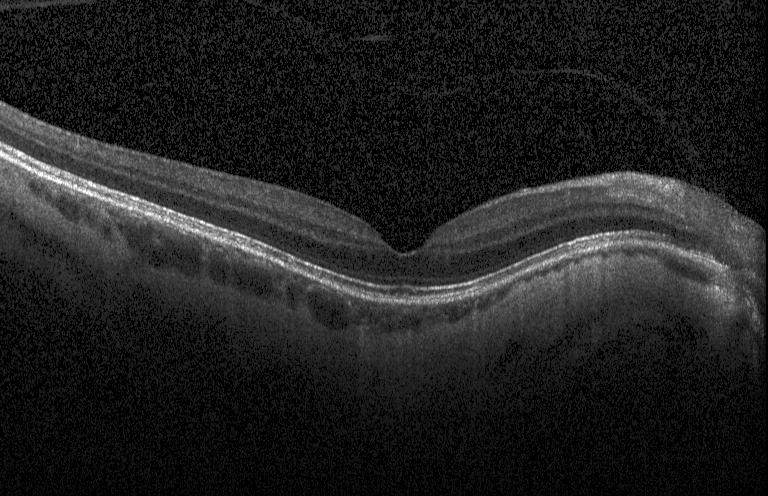 Spectral-domain optical coherence tomography · Heidelberg Spectralis · centered on the fovea · optical coherence tomography B-scan. Assessment: no choroidal neovascularization, no diabetic macular edema, and no drusen.